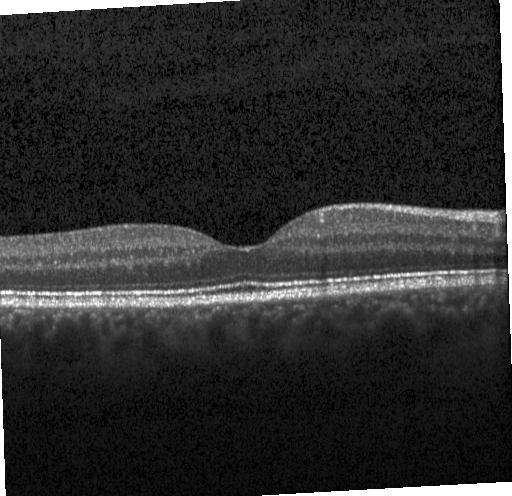

Spectral-domain OCT B-scan: no choroidal neovascularization, no diabetic macular edema, and no drusen.